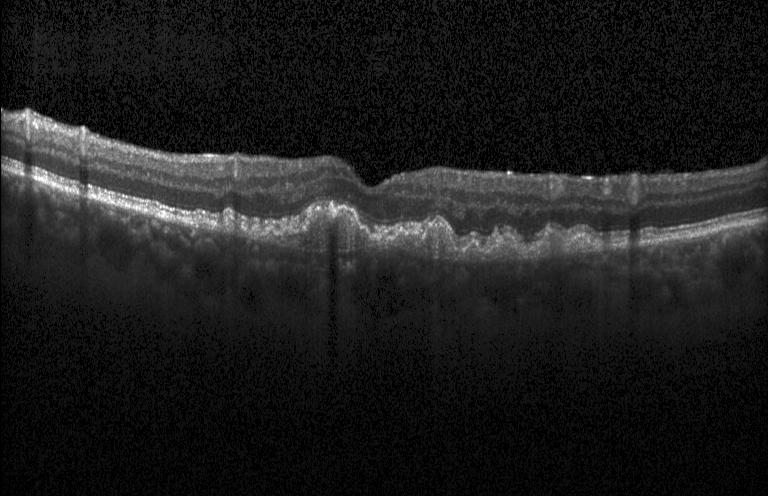 Spectral-domain optical coherence tomography. Heidelberg Spectralis. Retinal OCT B-scan — Impression: a choroidal neovascular membrane.